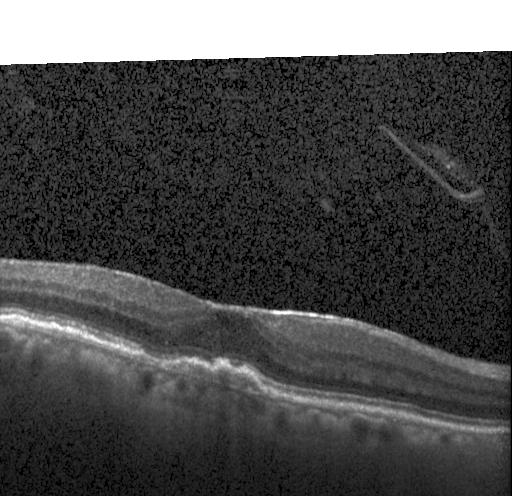

Optical coherence tomography B-scan.
The scan shows choroidal neovascularization (CNV).